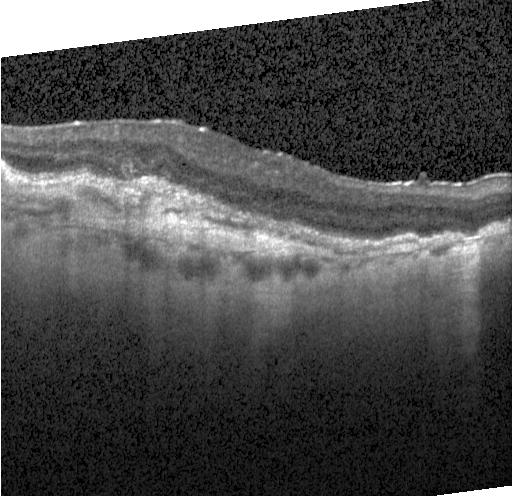

Macular OCT: a choroidal neovascular membrane.